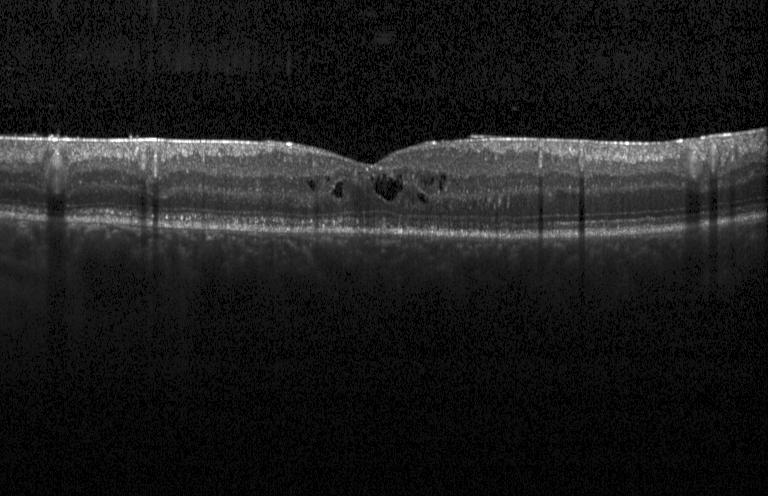 Macular OCT: DME.